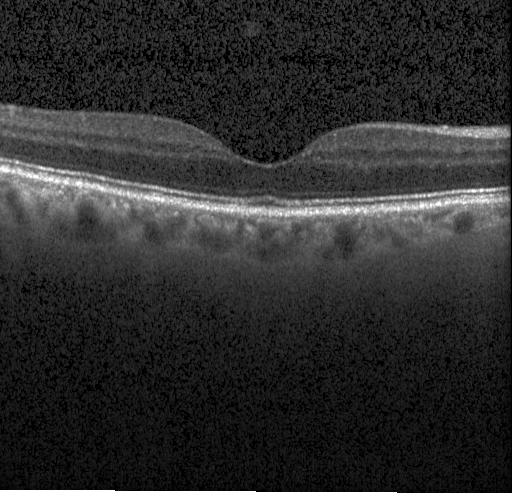

OCT B-scan.
The scan shows no choroidal neovascularization, no diabetic macular edema, and no drusen.